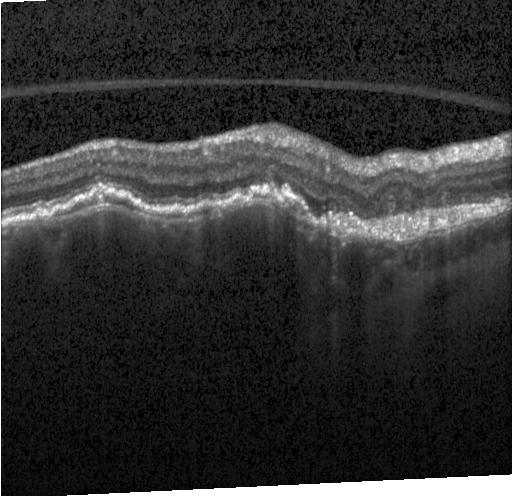
Spectral-domain OCT; retinal OCT B-scan. Diagnosis: choroidal neovascularization.